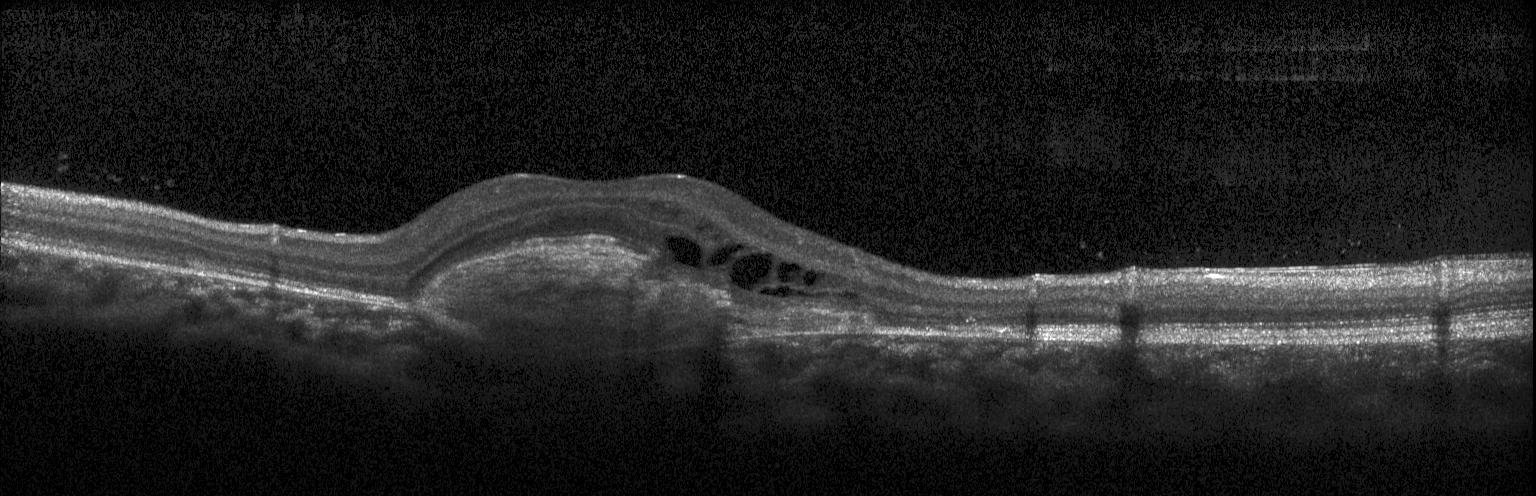

Impression: choroidal neovascularization (CNV).